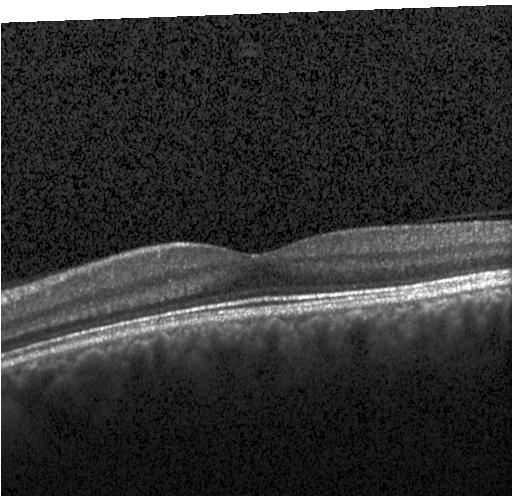

No CNV, DME, or drusen.